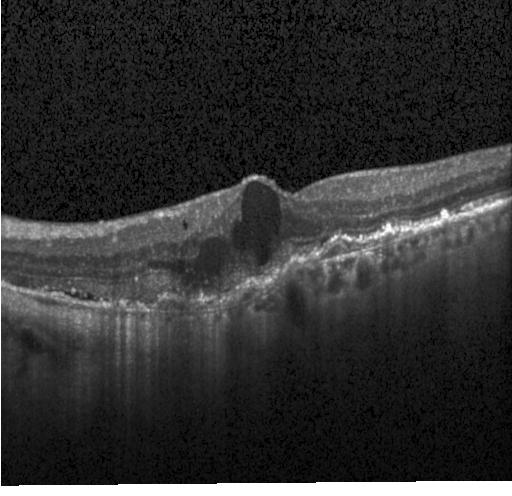

Horizontal scan through the fovea · retinal OCT cross-section · spectral-domain optical coherence tomography.
A choroidal neovascular membrane.